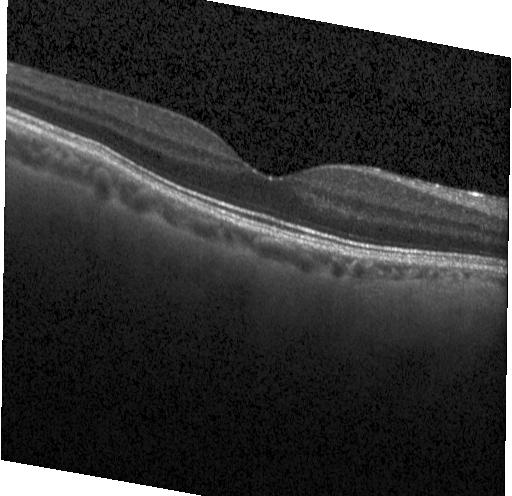 Optical coherence tomography scan
Diagnosis: no evidence of choroidal neovascularization, diabetic macular edema, or drusen.